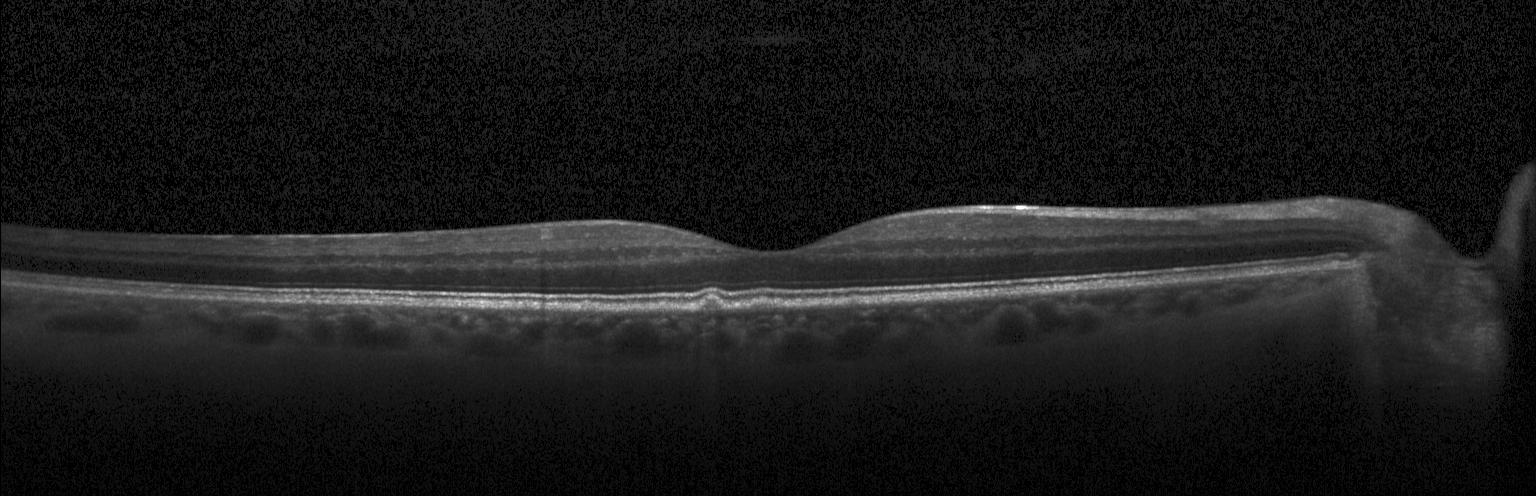 Horizontal scan through the fovea, spectral-domain optical coherence tomography, OCT line scan, Heidelberg Spectralis OCT system.
Diagnosis: multiple drusen.